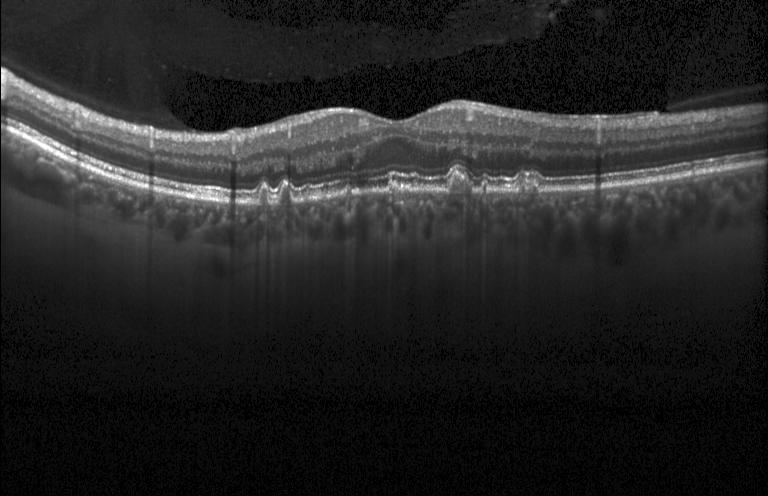 Spectral-domain OCT, optical coherence tomography scan, centered on the fovea, Heidelberg Spectralis OCT system — The scan shows drusen.